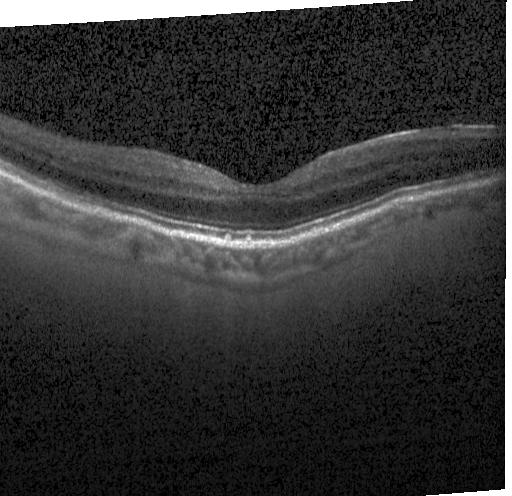
Heidelberg Spectralis OCT system · centered on the fovea · OCT B-scan · spectral-domain OCT
Impression: multiple drusen.